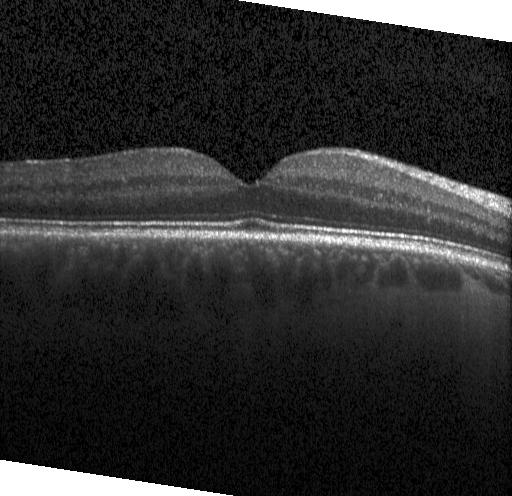

Impression: no choroidal neovascularization, no diabetic macular edema, and no drusen.